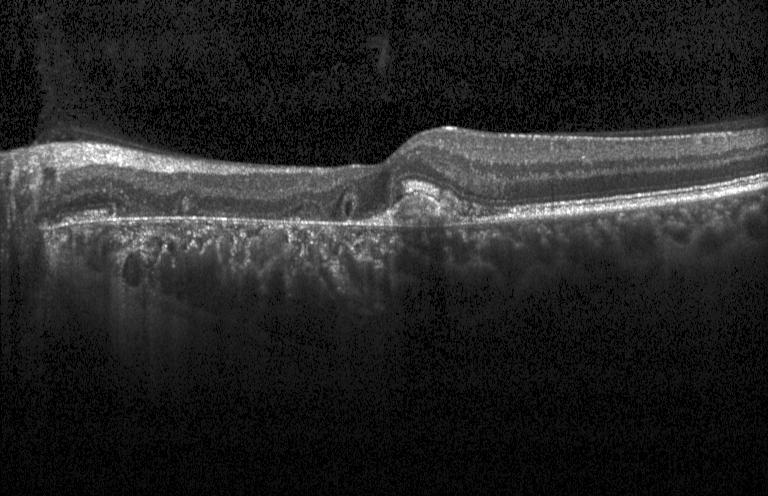

Diagnosis: choroidal neovascularization.